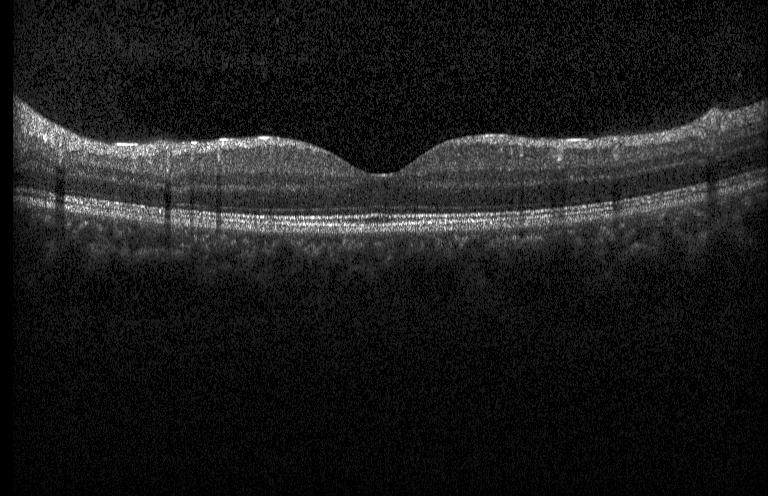 Finding: no choroidal neovascularization, no diabetic macular edema, and no drusen.